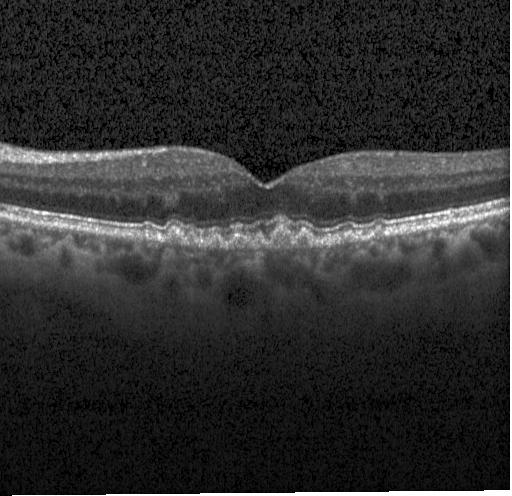
Fovea-centered; OCT line scan; spectral-domain OCT; acquired on a Heidelberg Spectralis
This B-scan demonstrates drusen.